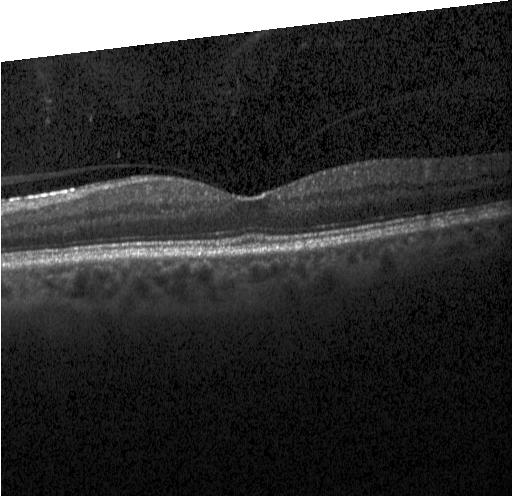
Spectral-domain OCT; acquired on a Heidelberg Spectralis; optical coherence tomography B-scan
Impression: no choroidal neovascularization, diabetic macular edema, or drusen.